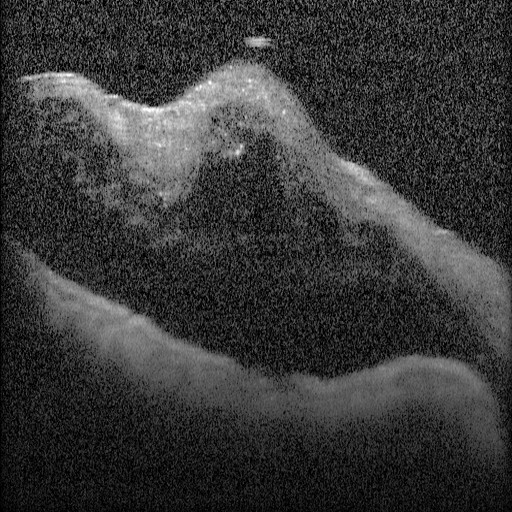

Retinal OCT cross-section.
Macular OCT: diabetic macular edema (DME).